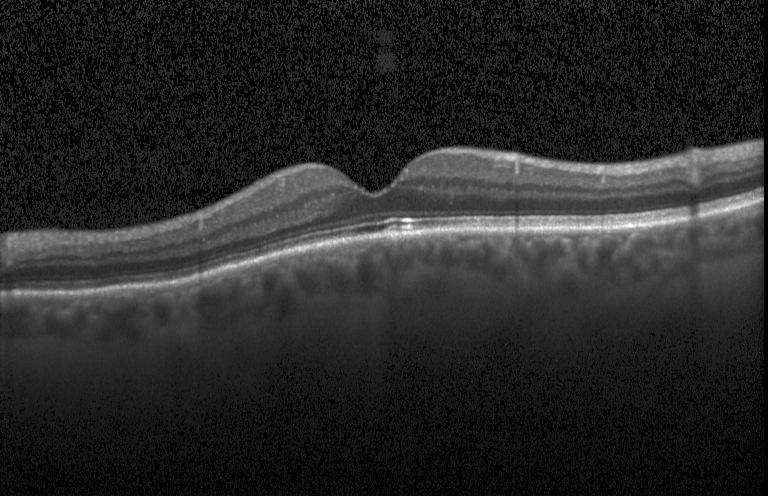

Finding: no choroidal neovascularization, no diabetic macular edema, and no drusen.